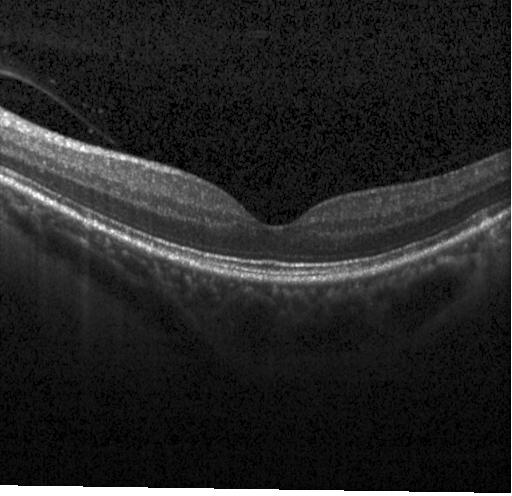 OCT finding: no choroidal neovascularization, diabetic macular edema, or drusen.